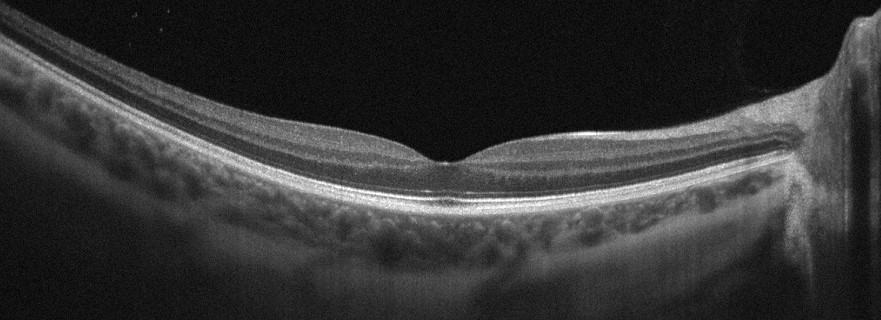

OCT B-scan; Optovue Avanti RTVue XR. Diagnosis: no evidence of AMD, DME, ERM, RAO, RVO, or VID.